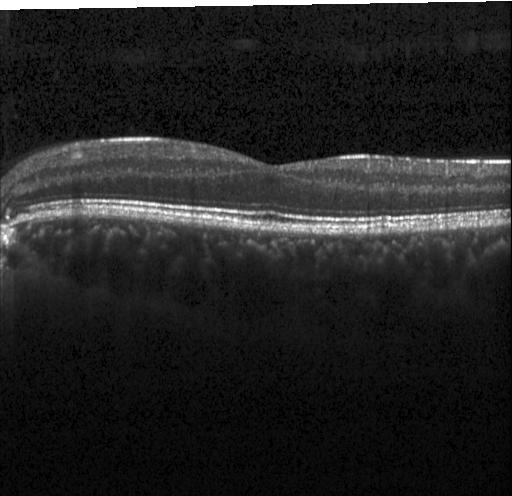
No choroidal neovascularization, no diabetic macular edema, and no drusen.